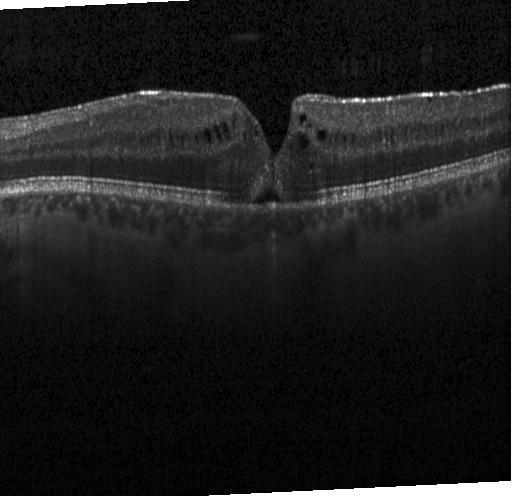
OCT line scan. Through the macula. Spectral-domain optical coherence tomography — OCT finding: diabetic macular edema.